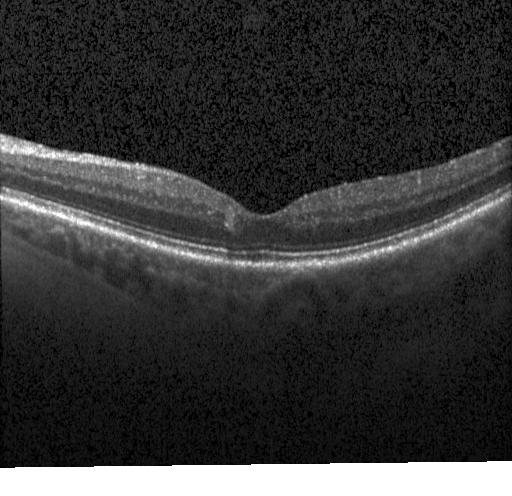

Dx: no CNV, no DME, and no drusen.